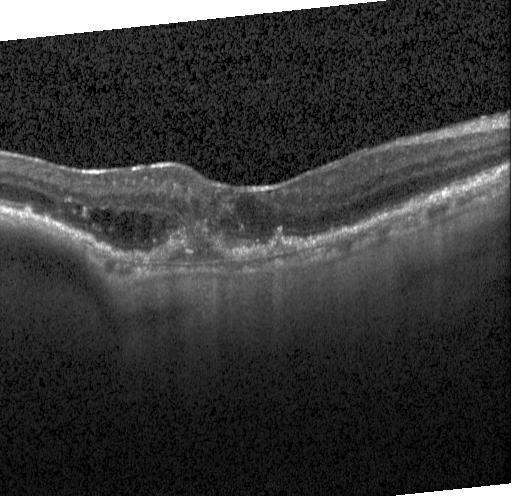

Diagnosis: a choroidal neovascular membrane.